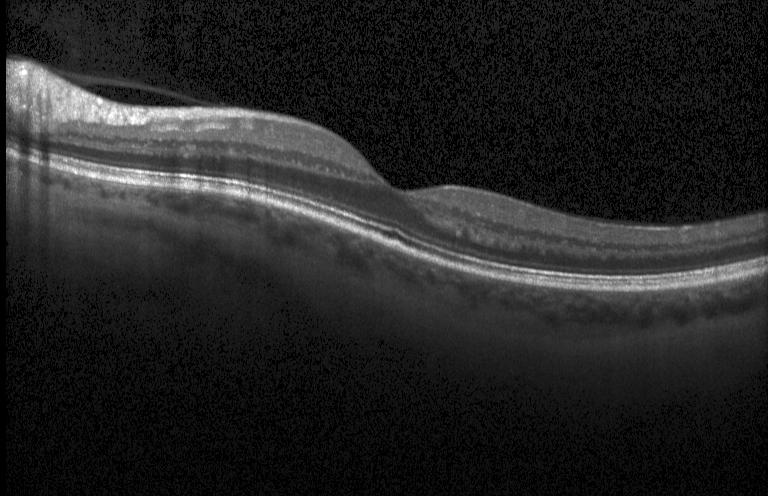 Optical coherence tomography B-scan — Diagnosis: no choroidal neovascularization, diabetic macular edema, or drusen.